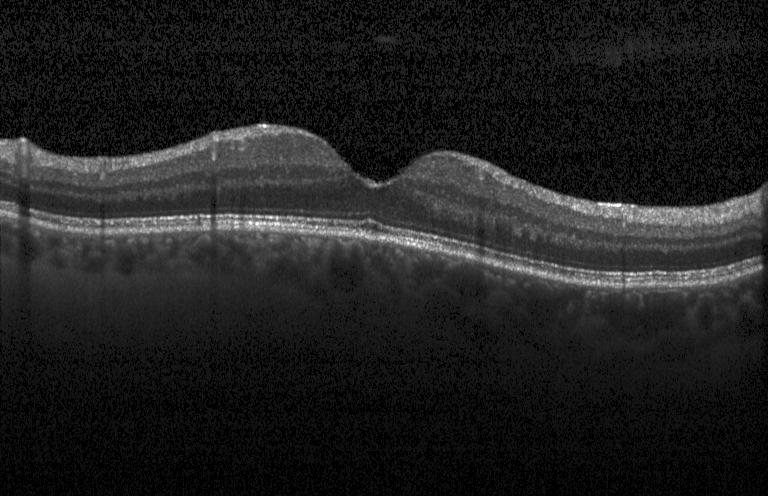
OCT B-scan. Horizontal scan through the fovea
Assessment: no evidence of choroidal neovascularization, diabetic macular edema, or drusen.